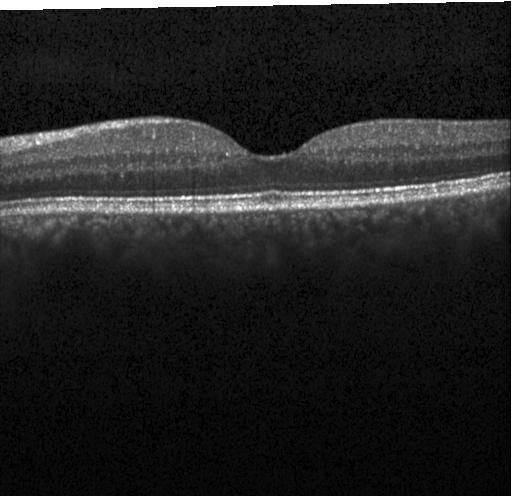
Horizontal scan through the fovea, instrument: Heidelberg Spectralis, optical coherence tomography scan.
No choroidal neovascularization, diabetic macular edema, or drusen.